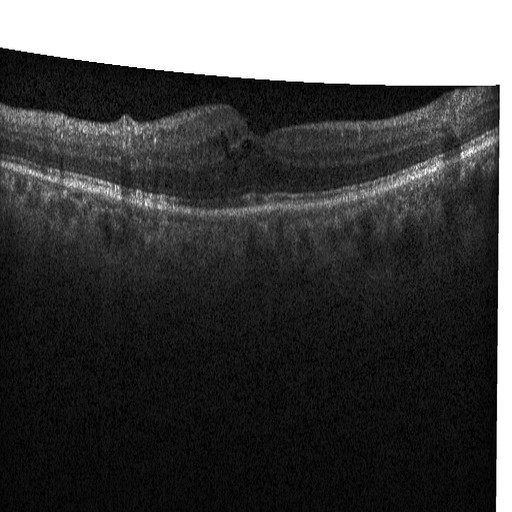
OCT line scan. Acquired on a Heidelberg Spectralis. Spectral-domain OCT. Finding: DME.